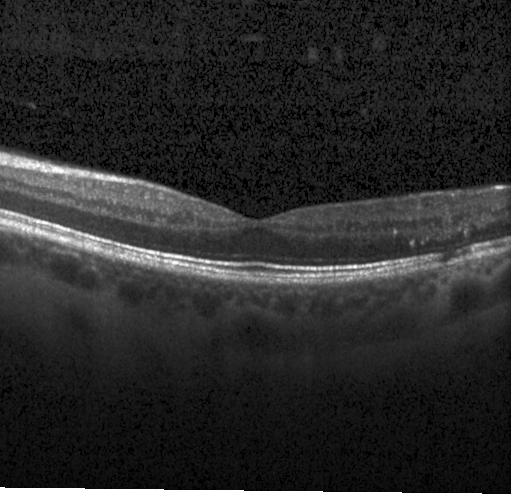
OCT scan showing no CNV, no DME, and no drusen.